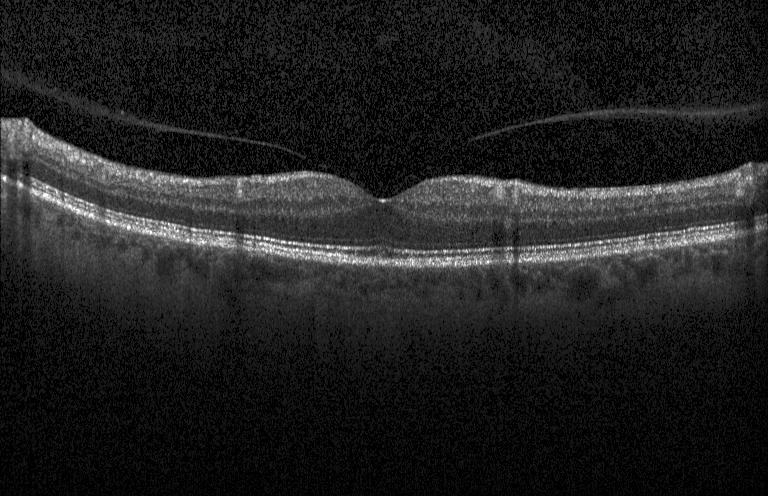
OCT line scan · acquired on a Heidelberg Spectralis · fovea-centered — The scan shows no choroidal neovascularization, diabetic macular edema, or drusen.